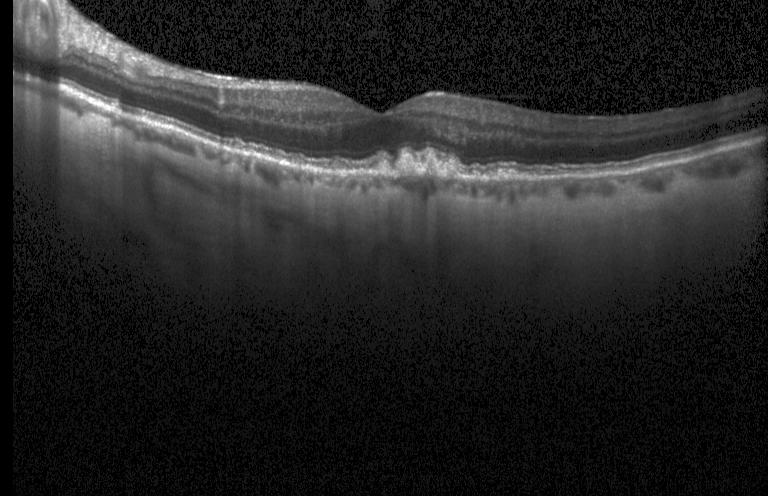

OCT B-scan. Diagnosis: sub-RPE drusenoid deposits.